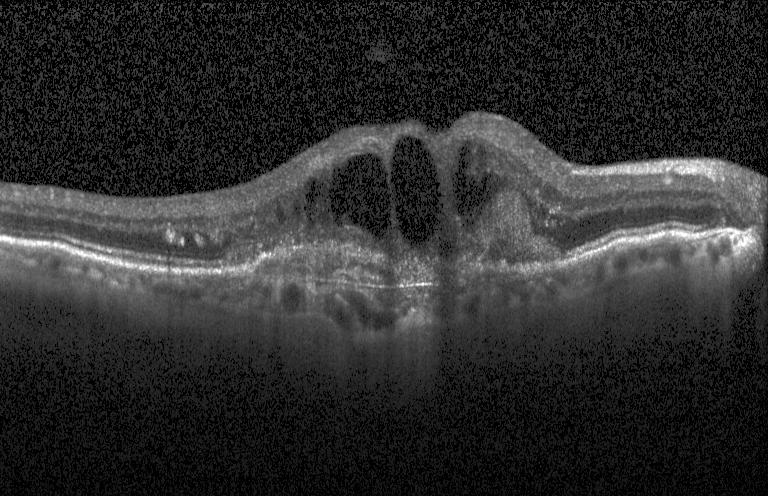

Optical coherence tomography scan · SD-OCT · instrument: Heidelberg Spectralis · horizontal scan through the fovea. Impression: a choroidal neovascular membrane.